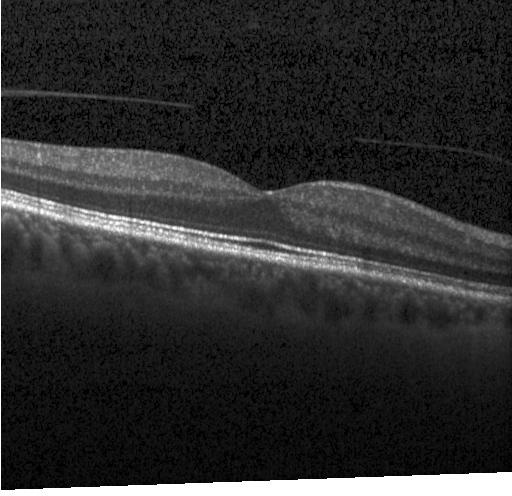 This B-scan demonstrates neither CNV, DME, nor drusen.